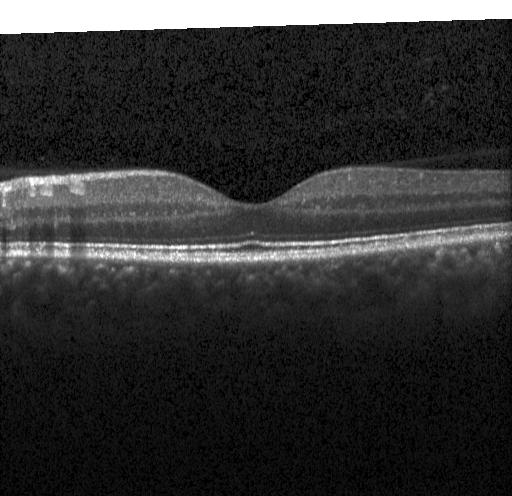
Finding: no choroidal neovascularization, diabetic macular edema, or drusen.